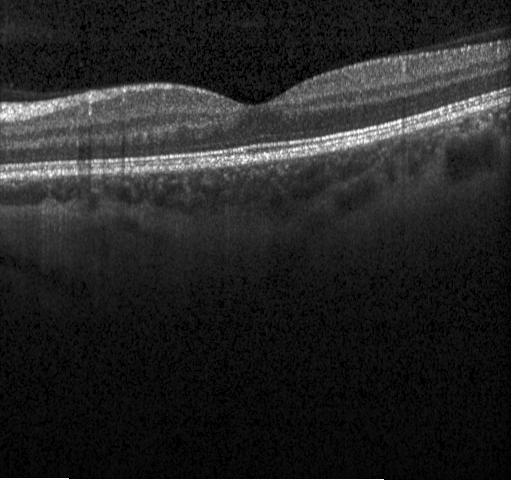

Fovea-centered; retinal OCT cross-section. This B-scan demonstrates no CNV, DME, or drusen.